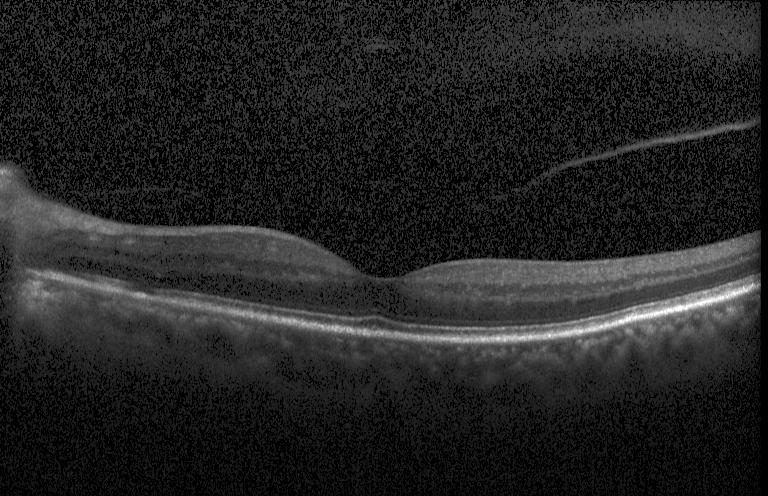
OCT B-scan.
Impression: no evidence of choroidal neovascularization, diabetic macular edema, or drusen.